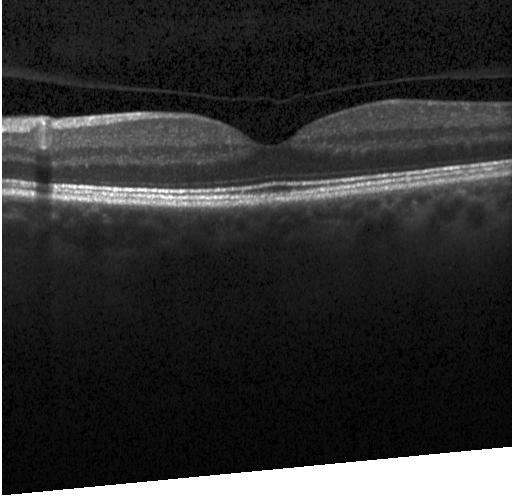
OCT B-scan.
Assessment: no choroidal neovascularization, diabetic macular edema, or drusen.